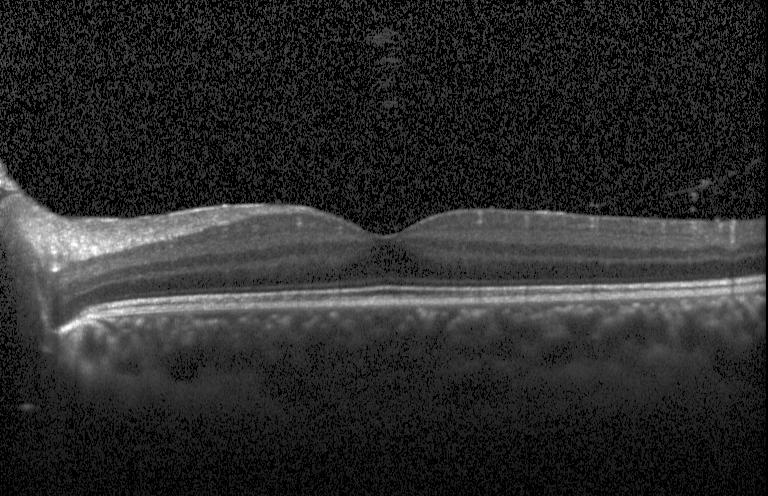
Diagnosis: no choroidal neovascularization, diabetic macular edema, or drusen.